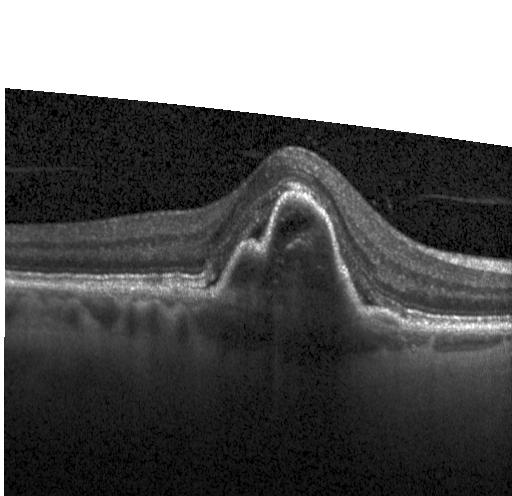

Optical coherence tomography B-scan; horizontal scan through the fovea; spectral-domain OCT
A choroidal neovascular membrane.